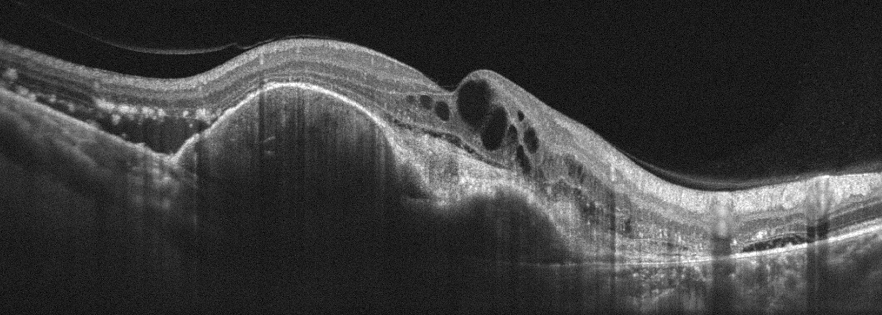 Finding: AMD.